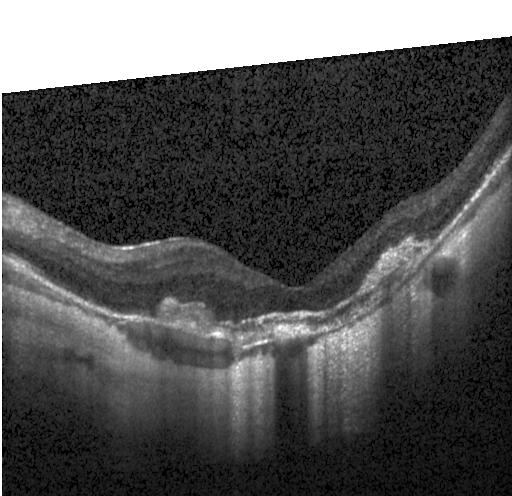

Retinal OCT B-scan
This B-scan demonstrates choroidal neovascularization (CNV).